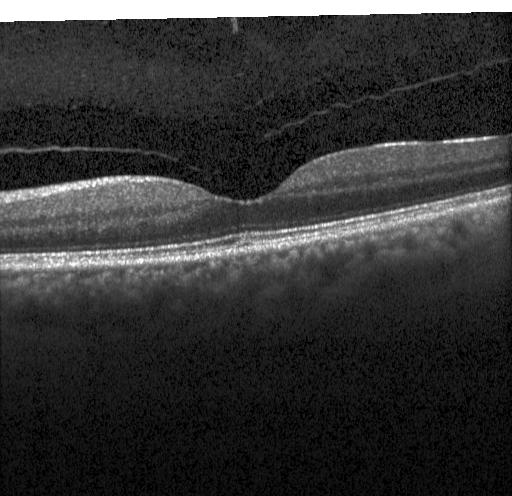
Dx: neither choroidal neovascularization, diabetic macular edema, nor drusen.